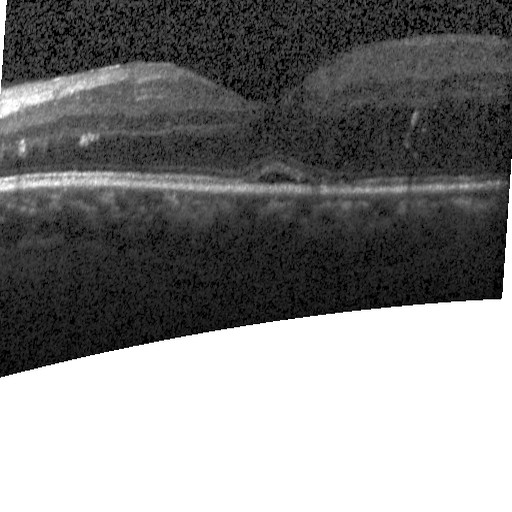 Acquired on a Heidelberg Spectralis, optical coherence tomography scan.
The scan shows DME.